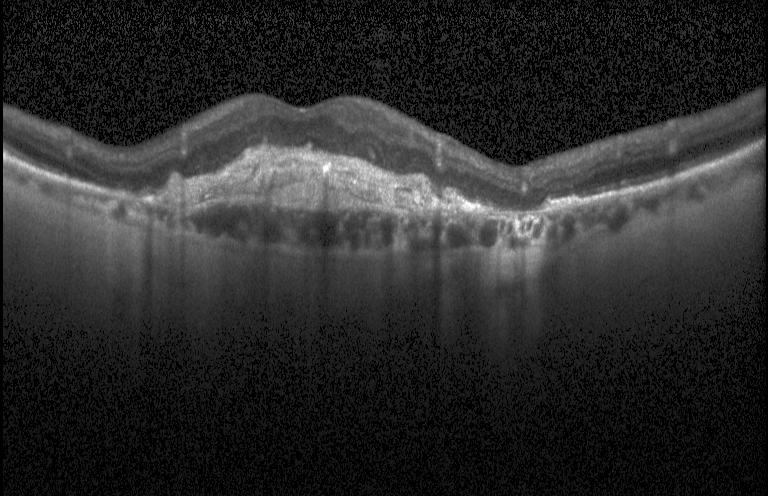
Optical coherence tomography scan
Finding: choroidal neovascularization.